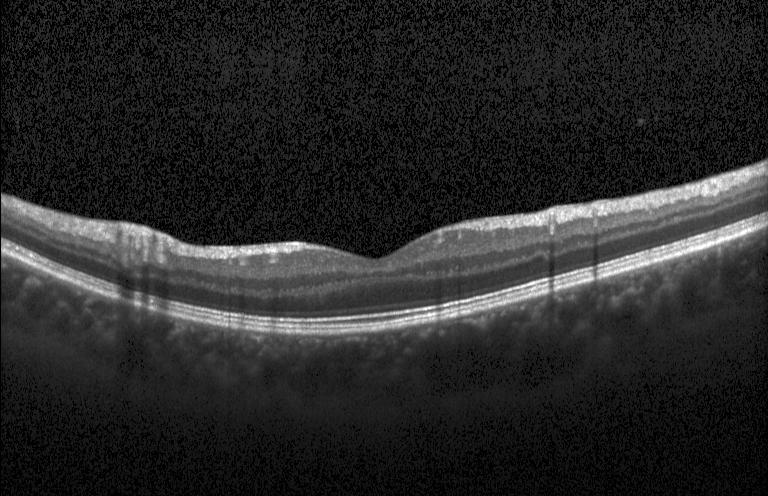
Macular scan; retinal OCT B-scan; instrument: Heidelberg Spectralis — Finding: neither choroidal neovascularization, diabetic macular edema, nor drusen.